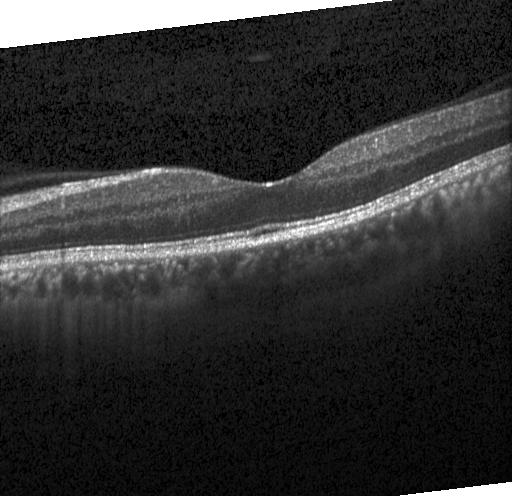 Heidelberg Spectralis, optical coherence tomography scan — No CNV, no DME, and no drusen.